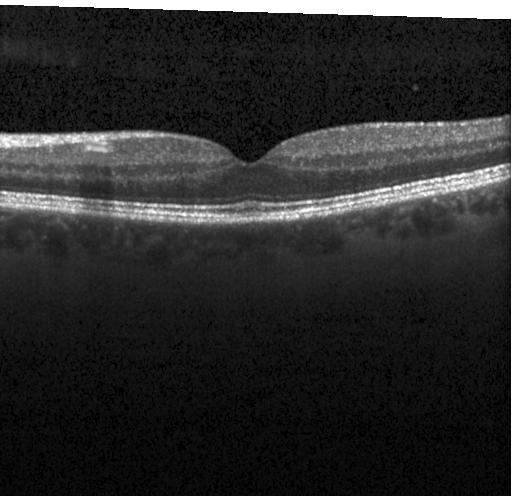

OCT scan showing no evidence of choroidal neovascularization, diabetic macular edema, or drusen.